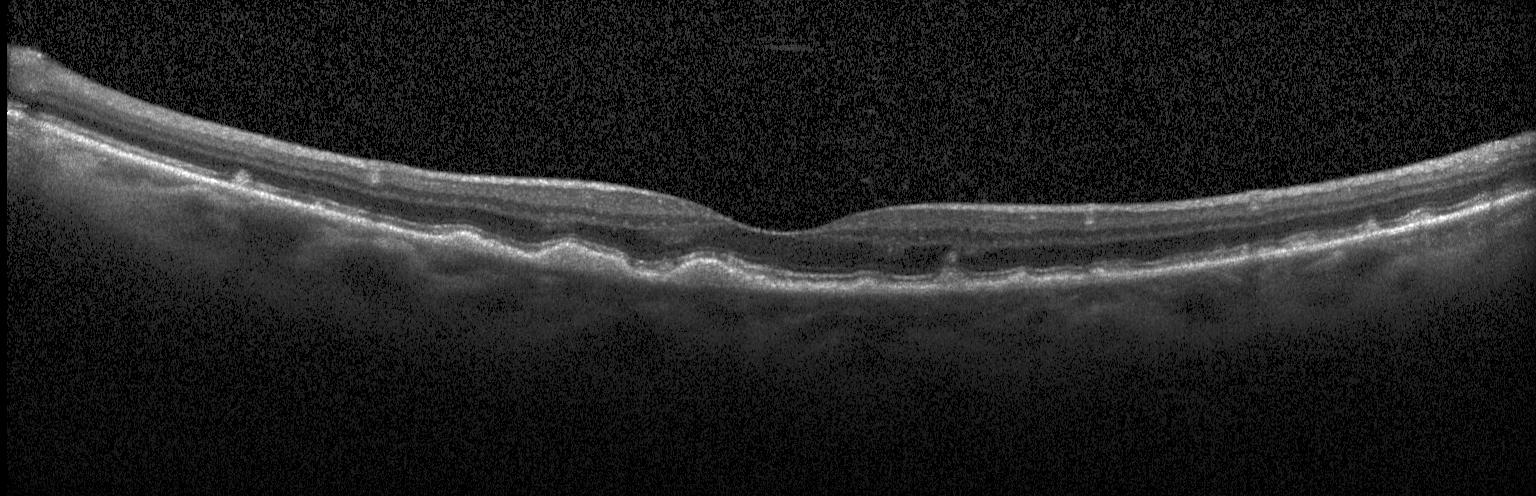

This B-scan demonstrates multiple drusen.